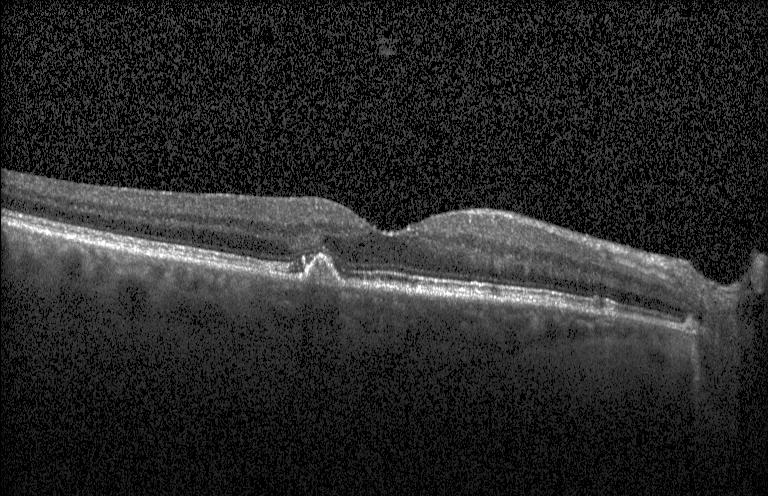
Optical coherence tomography scan; SD-OCT; horizontal scan through the fovea; Heidelberg Spectralis OCT system — Assessment: choroidal neovascularization (CNV).